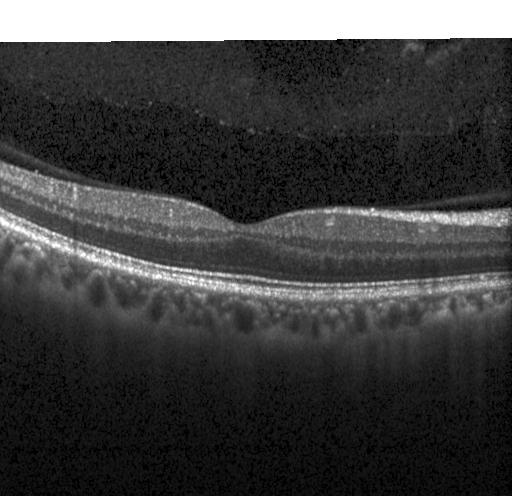

Centered on the fovea. Heidelberg Spectralis OCT system. OCT line scan
Assessment: no choroidal neovascularization, diabetic macular edema, or drusen.